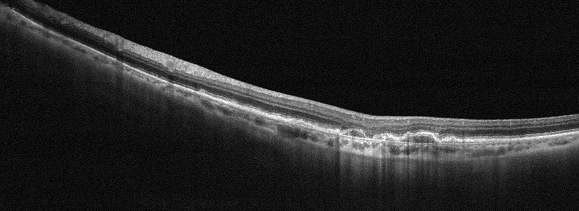

Oculus sinister, optical coherence tomography scan. Diagnosis: age-related macular degeneration (AMD).